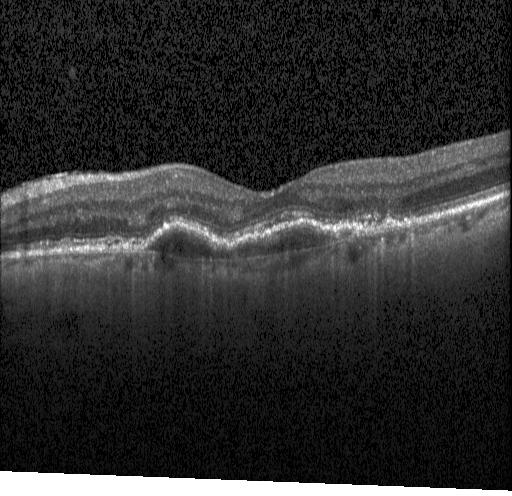
OCT line scan. SD-OCT. Impression: a choroidal neovascular membrane.